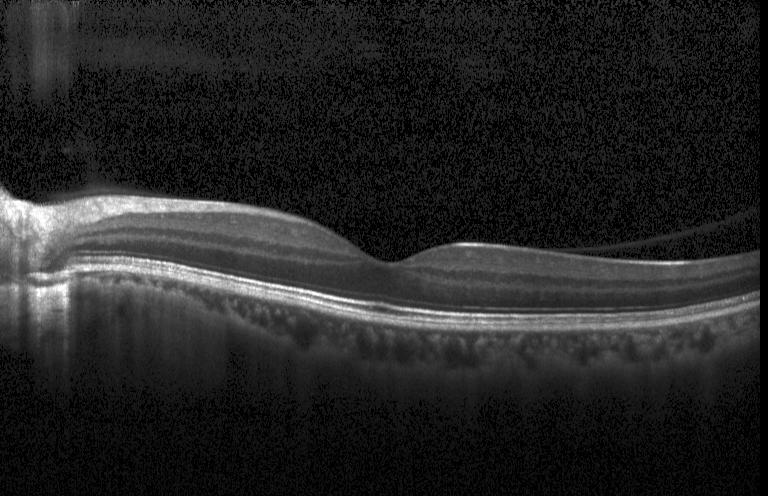

Assessment: neither choroidal neovascularization, diabetic macular edema, nor drusen.